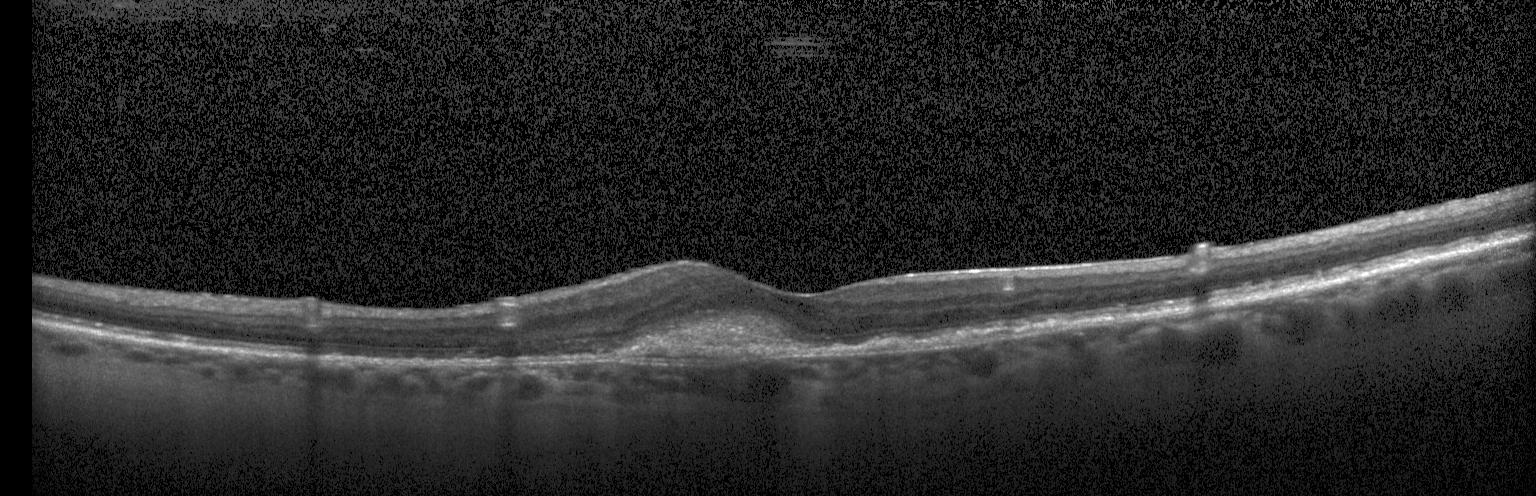
Centered on the fovea, optical coherence tomography B-scan — OCT finding: a choroidal neovascular membrane.